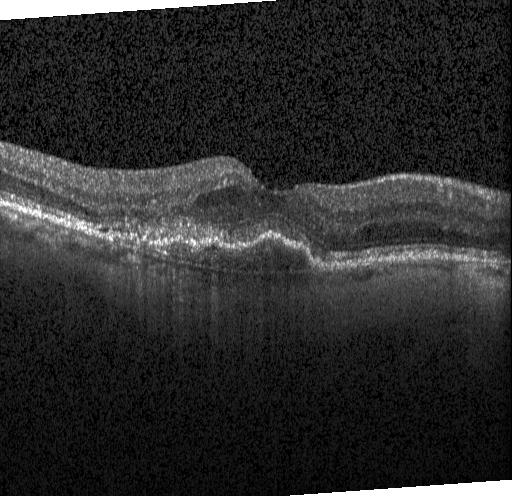 Dx: a choroidal neovascular membrane.